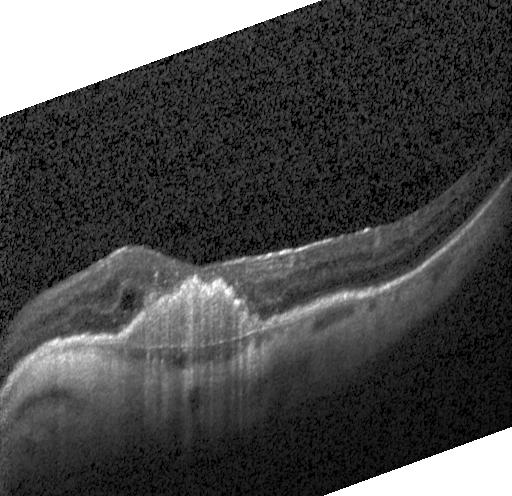
OCT B-scan — Finding: a choroidal neovascular membrane.